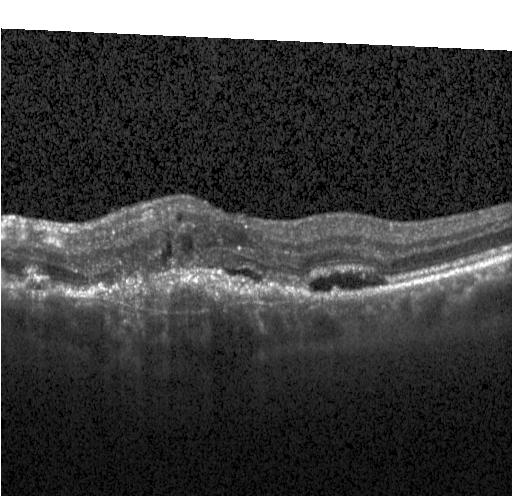
Through the macula; OCT line scan; spectral-domain optical coherence tomography; Heidelberg Spectralis
This B-scan demonstrates a choroidal neovascular membrane.